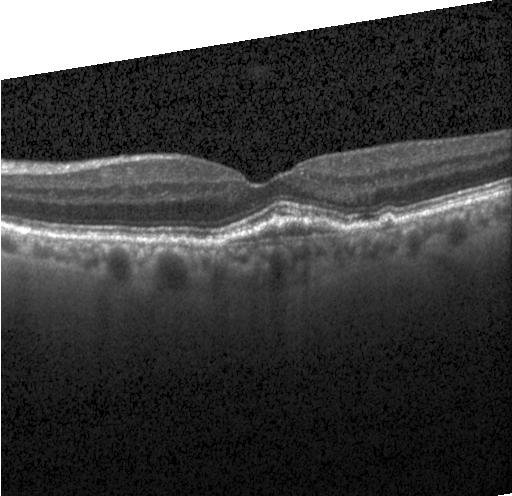
Centered on the fovea, instrument: Heidelberg Spectralis, OCT line scan, spectral-domain OCT.
The scan shows CNV.